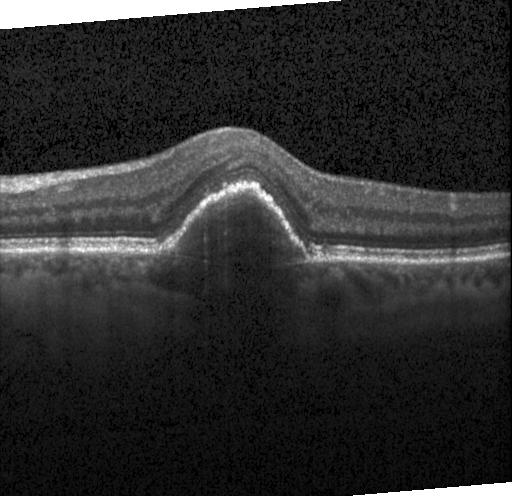

OCT B-scan.
This B-scan demonstrates a choroidal neovascular membrane.